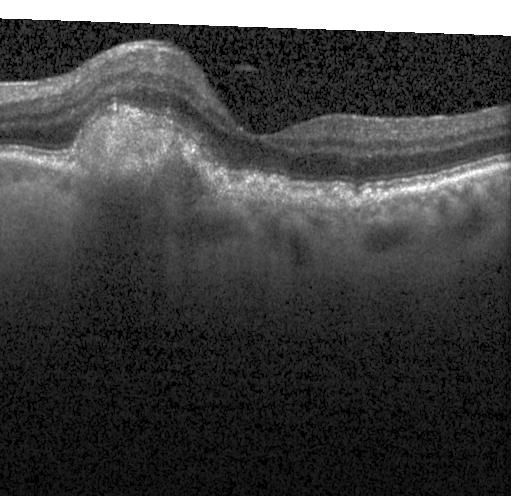 Diagnosis: choroidal neovascularization (CNV).